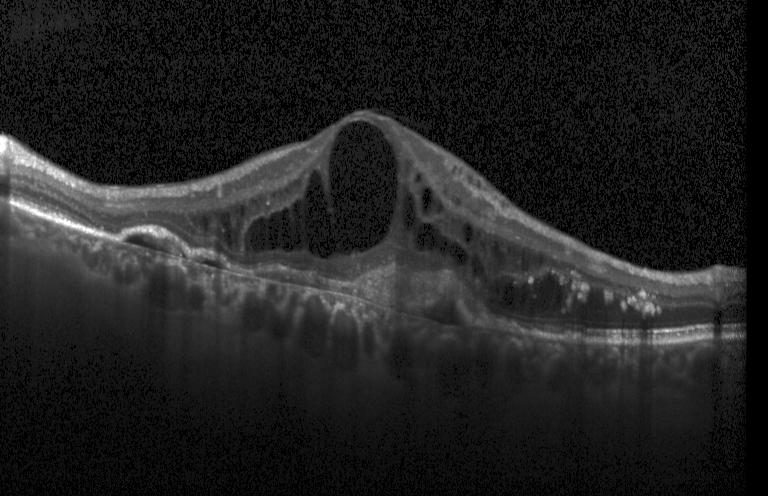
Assessment: a choroidal neovascular membrane.